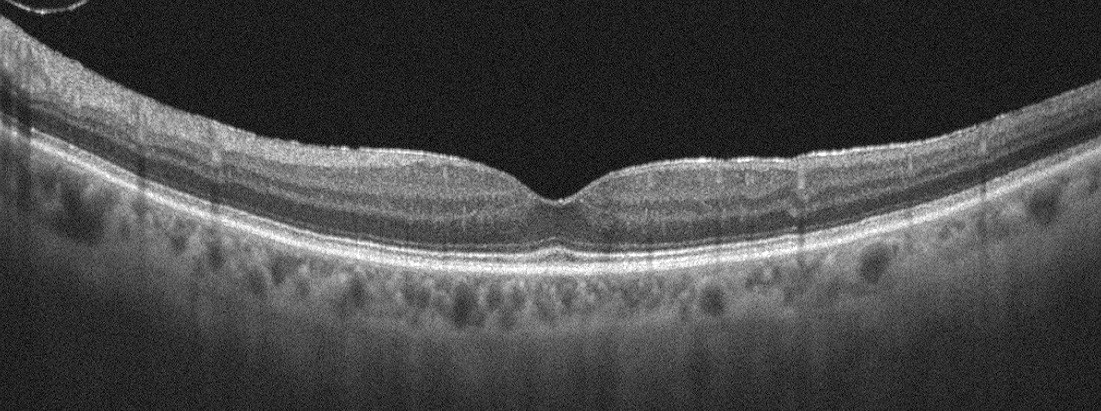 Retinal OCT cross-section. Assessment: ERM.